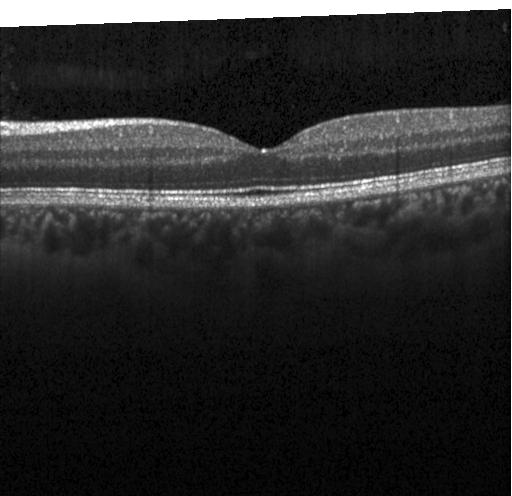
Diagnosis: no evidence of choroidal neovascularization, diabetic macular edema, or drusen.